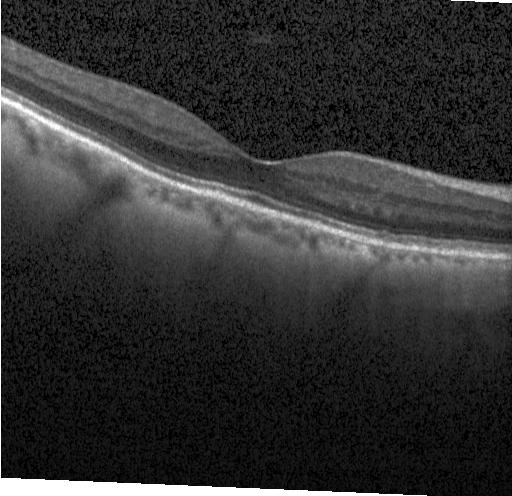
OCT B-scan · Heidelberg Spectralis OCT system · spectral-domain OCT.
Neither choroidal neovascularization, diabetic macular edema, nor drusen.